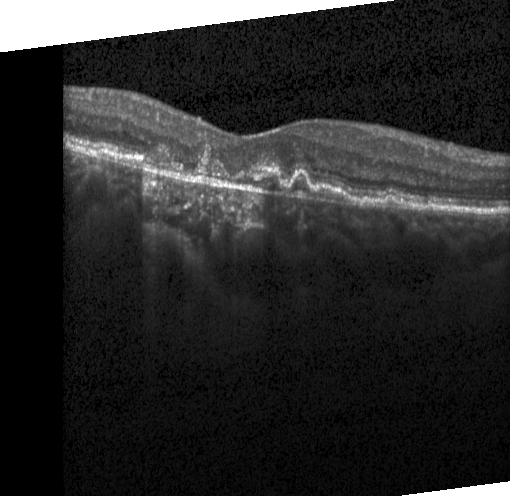
Retinal OCT cross-section showing choroidal neovascularization.